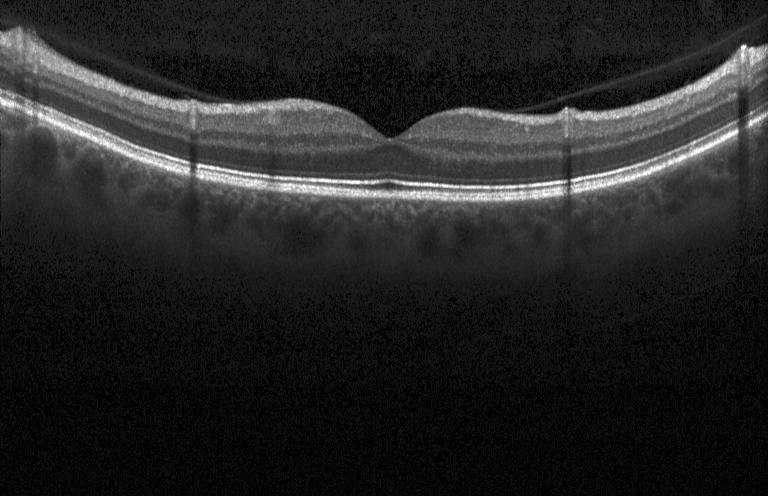 Spectral-domain OCT B-scan: neither CNV, DME, nor drusen.